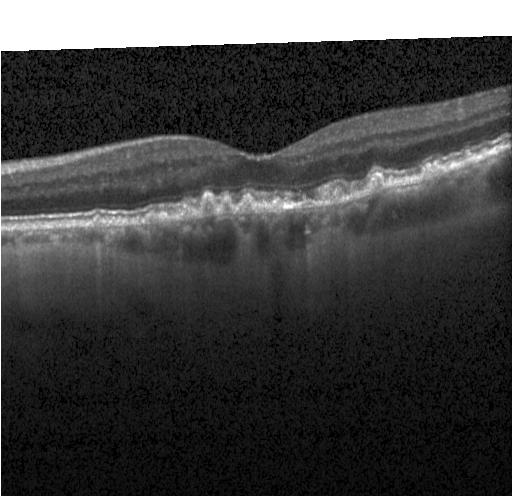

Retinal OCT B-scan; horizontal scan through the fovea. Diagnosis: multiple drusen.